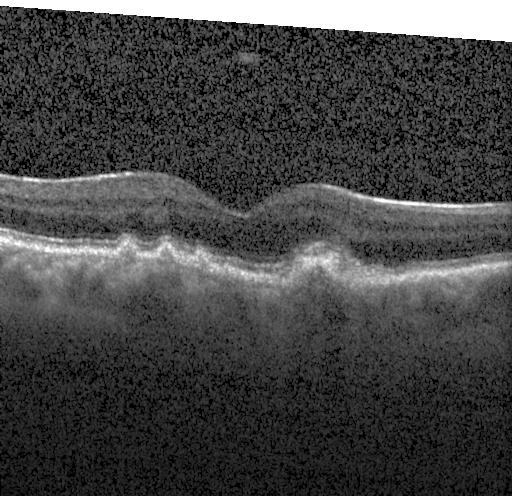
SD-OCT. Fovea-centered. OCT line scan. Instrument: Heidelberg Spectralis — Dx: drusen.